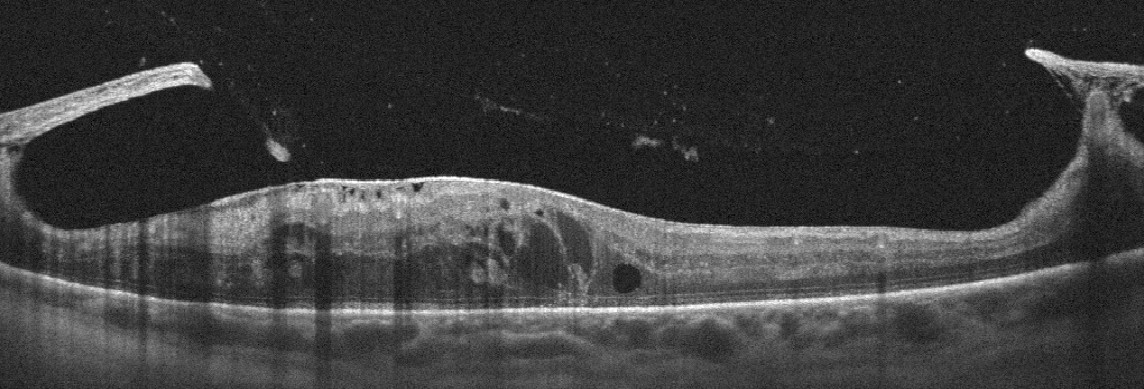

Acquired on an Optovue Avanti RTVue XR. Retinal OCT B-scan
Diagnosis: diabetic macular edema (DME).